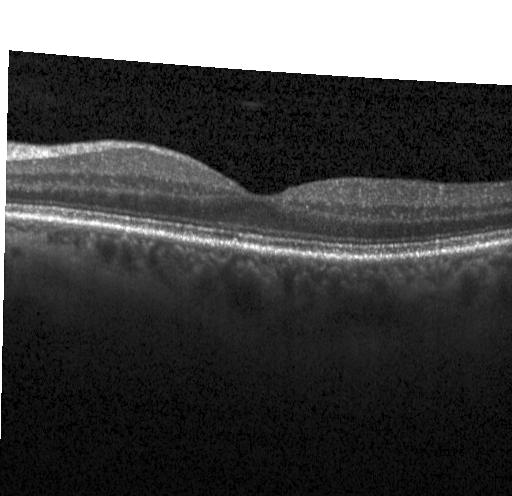
Optical coherence tomography scan. Macular OCT: no choroidal neovascularization, no diabetic macular edema, and no drusen.